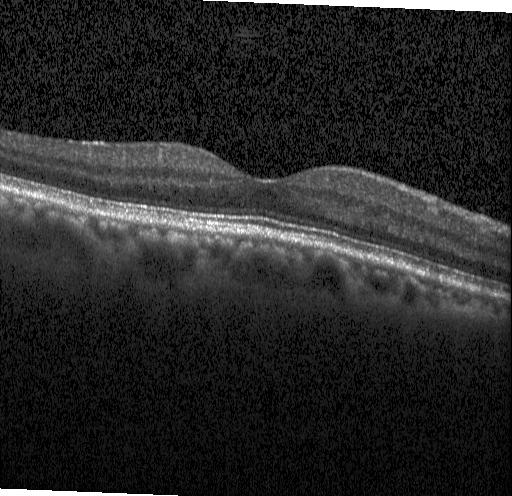
Centered on the fovea; spectral-domain OCT; OCT B-scan. Finding: no choroidal neovascularization, no diabetic macular edema, and no drusen.